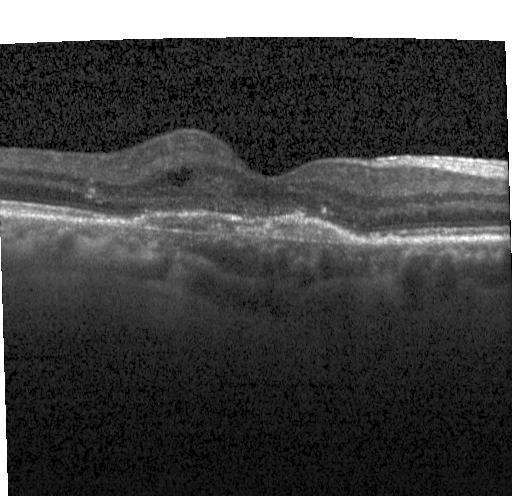
Macular scan. Heidelberg Spectralis. Retinal OCT cross-section. Diagnosis: a choroidal neovascular membrane.